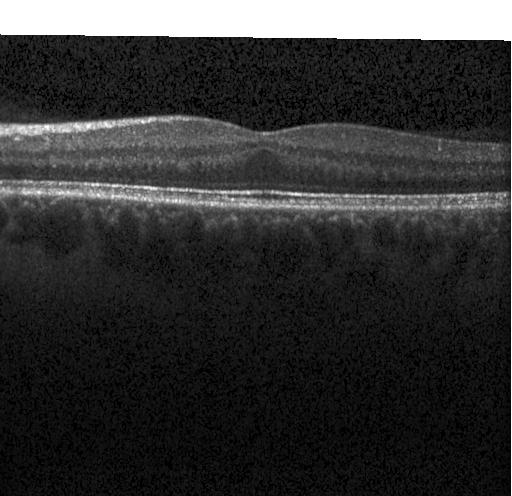
OCT line scan, Heidelberg Spectralis.
Dx: neither choroidal neovascularization, diabetic macular edema, nor drusen.